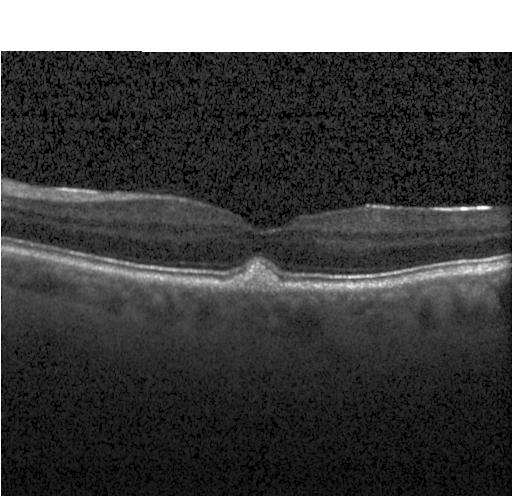
SD-OCT. OCT line scan
Impression: sub-RPE drusenoid deposits.